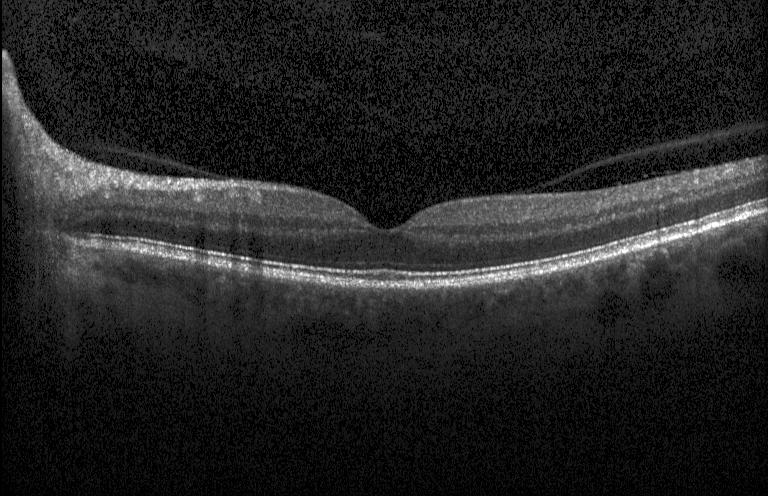 Horizontal scan through the fovea, optical coherence tomography B-scan — Impression: no evidence of CNV, DME, or drusen.